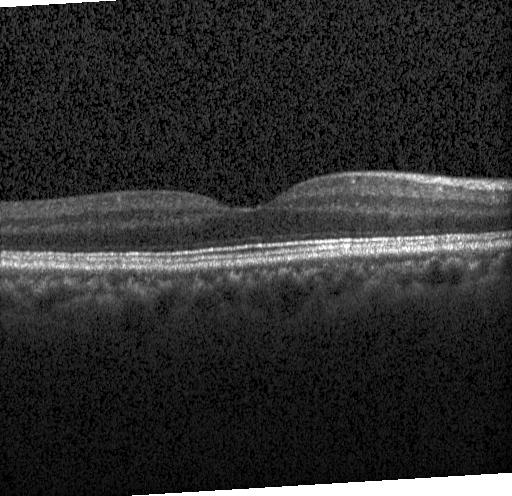

Heidelberg Spectralis; OCT B-scan
Diagnosis: no evidence of CNV, DME, or drusen.